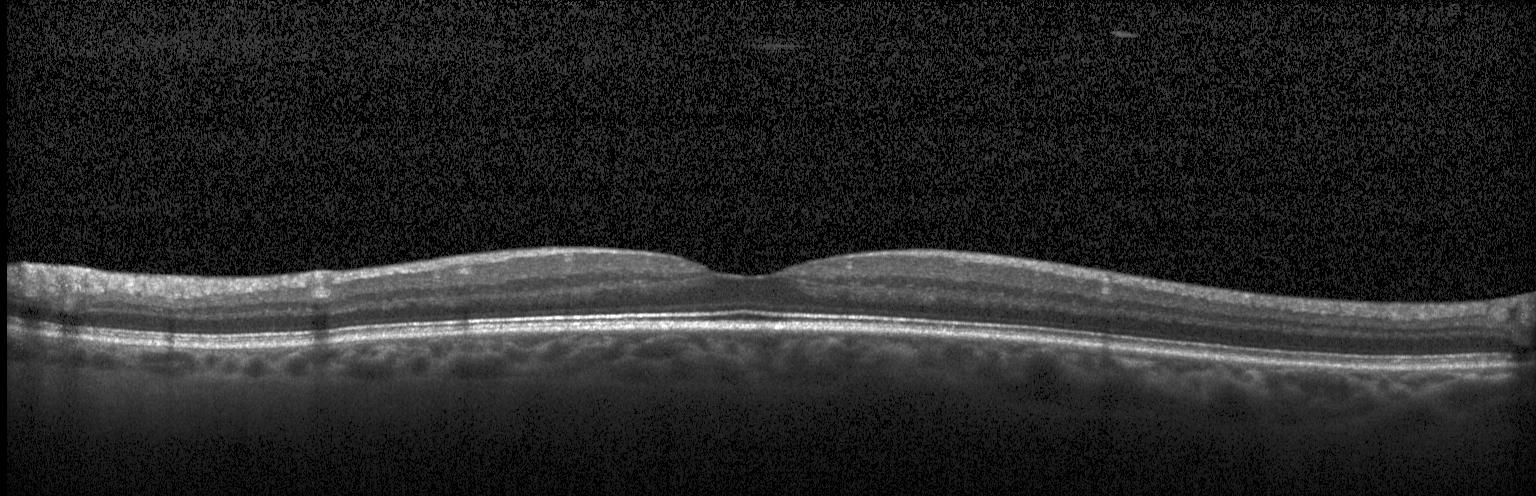

Macular OCT: neither CNV, DME, nor drusen.